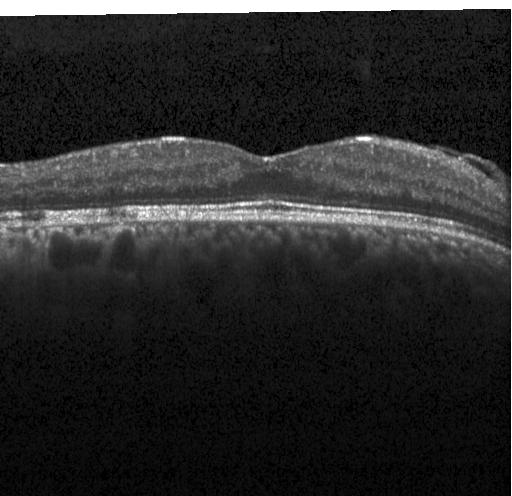

Retinal OCT B-scan. Spectral-domain optical coherence tomography. Acquired on a Heidelberg Spectralis. Horizontal scan through the fovea
Diagnosis: no CNV, DME, or drusen.